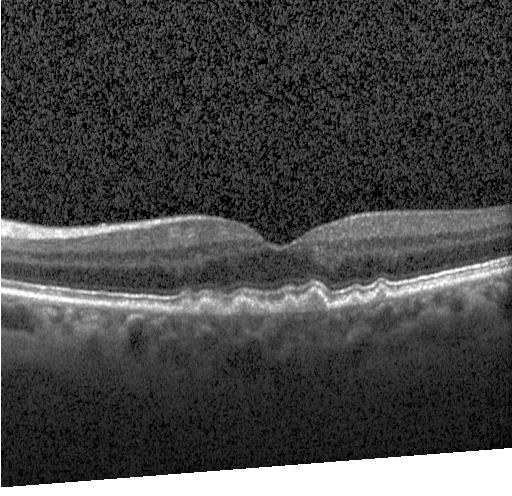
Assessment: sub-RPE drusenoid deposits.